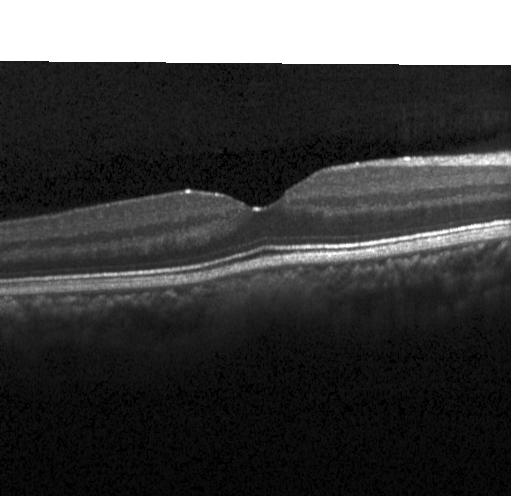 Retinal OCT cross-section. Dx: no choroidal neovascularization, diabetic macular edema, or drusen.